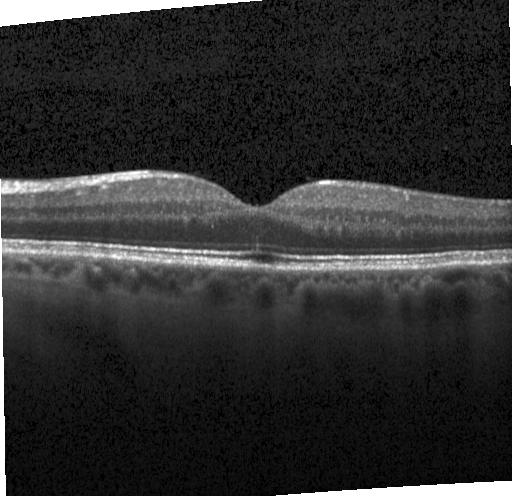 Diagnosis: no choroidal neovascularization, diabetic macular edema, or drusen.